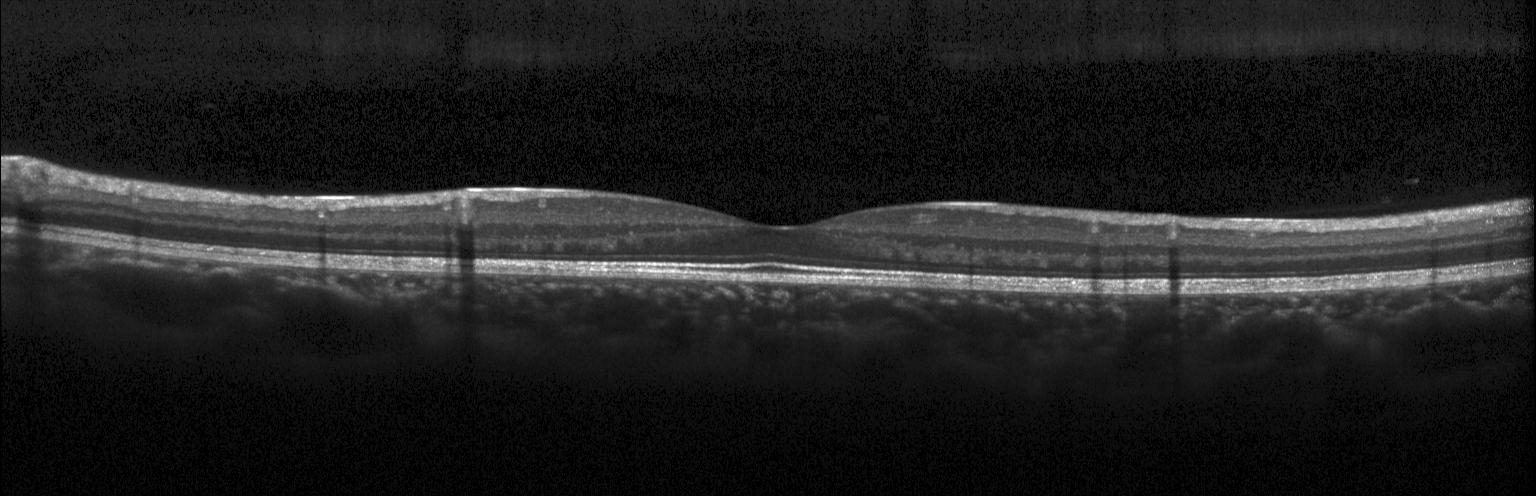 Spectral-domain optical coherence tomography, macular scan, retinal OCT B-scan, Heidelberg Spectralis.
Diagnosis: no choroidal neovascularization, diabetic macular edema, or drusen.